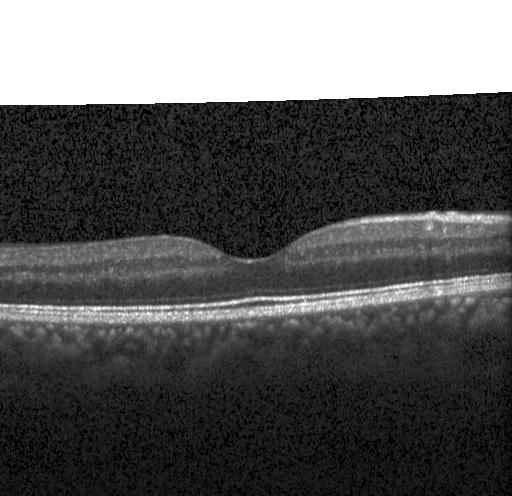

Through the macula · Heidelberg Spectralis · optical coherence tomography scan.
No choroidal neovascularization, diabetic macular edema, or drusen.